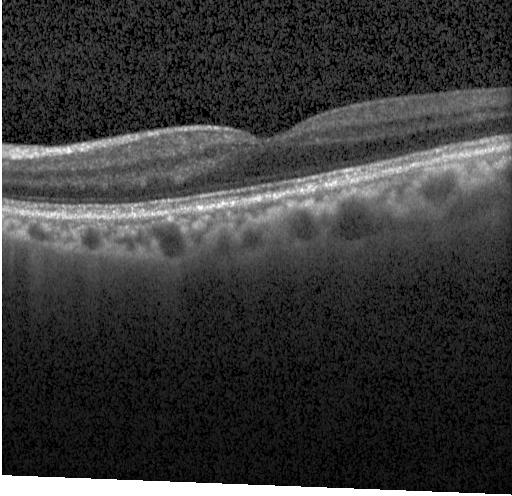

Acquired on a Heidelberg Spectralis; horizontal scan through the fovea; optical coherence tomography scan; spectral-domain OCT. Impression: neither choroidal neovascularization, diabetic macular edema, nor drusen.